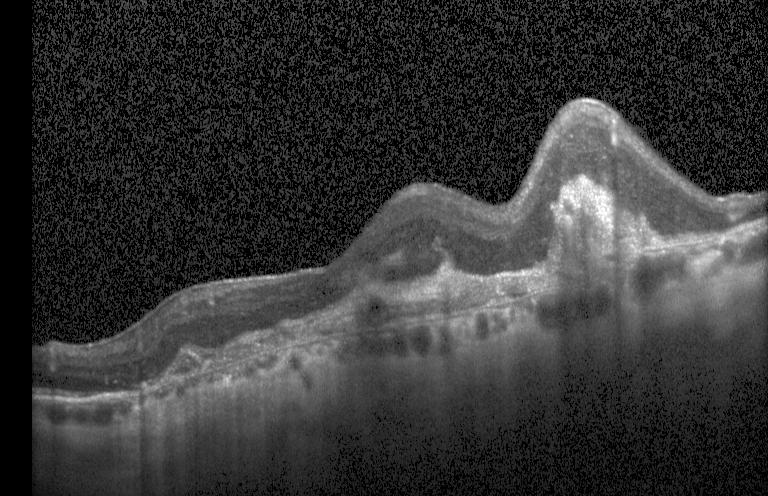 OCT B-scan. Centered on the fovea
Dx: a choroidal neovascular membrane.